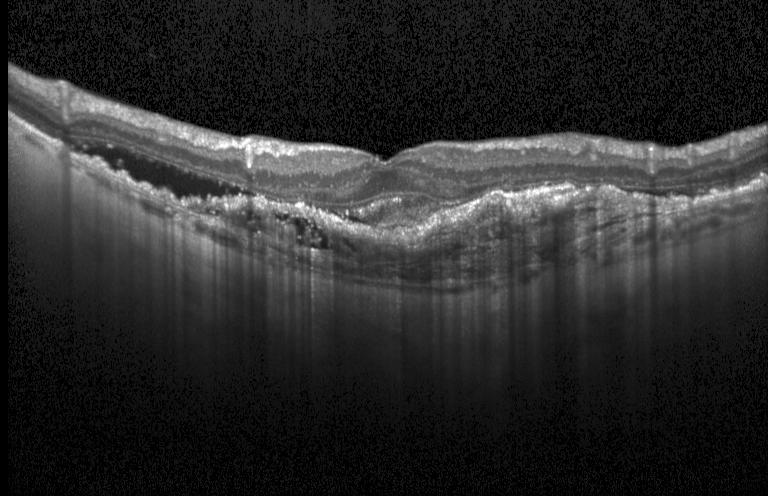

Macular OCT demonstrating a choroidal neovascular membrane.